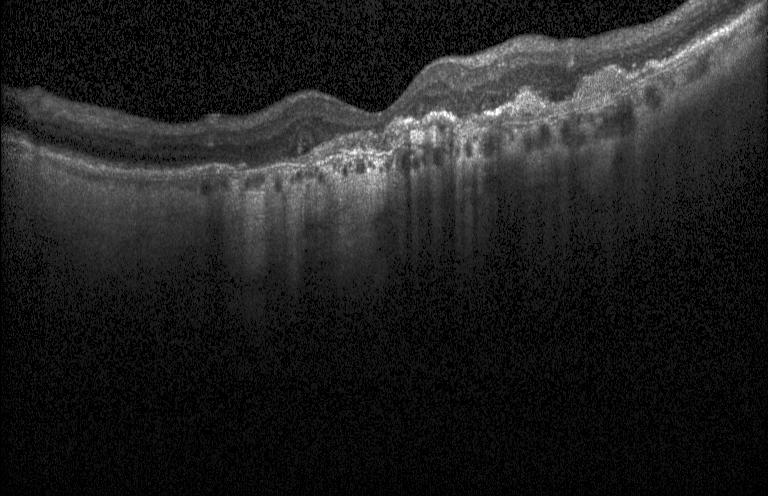
OCT B-scan showing a choroidal neovascular membrane.